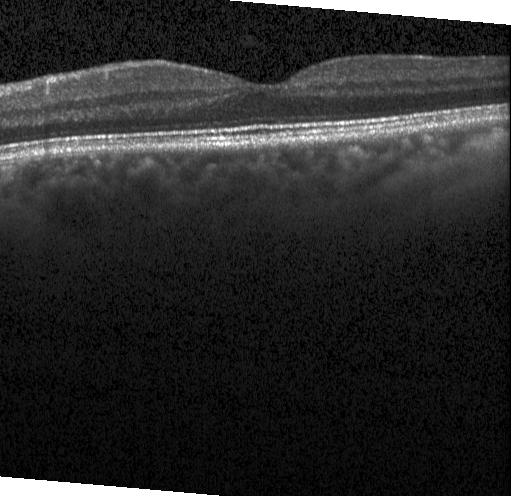
Macular OCT: neither CNV, DME, nor drusen.